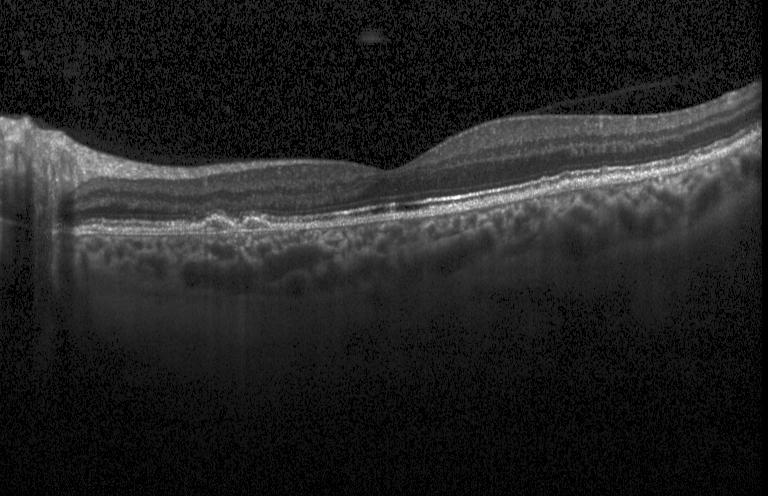

OCT B-scan — Diagnosis: choroidal neovascularization.